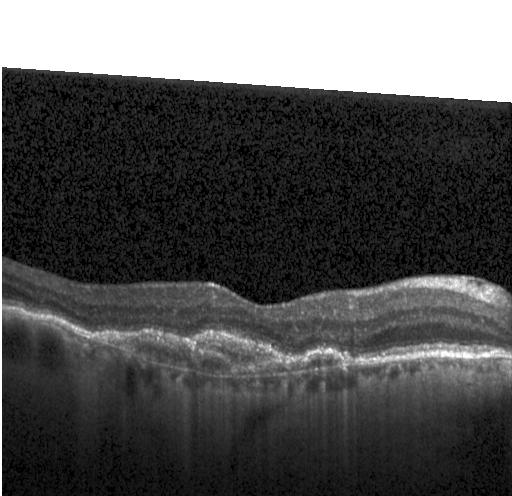 Optical coherence tomography B-scan, SD-OCT, instrument: Heidelberg Spectralis, macular scan — Impression: a choroidal neovascular membrane.